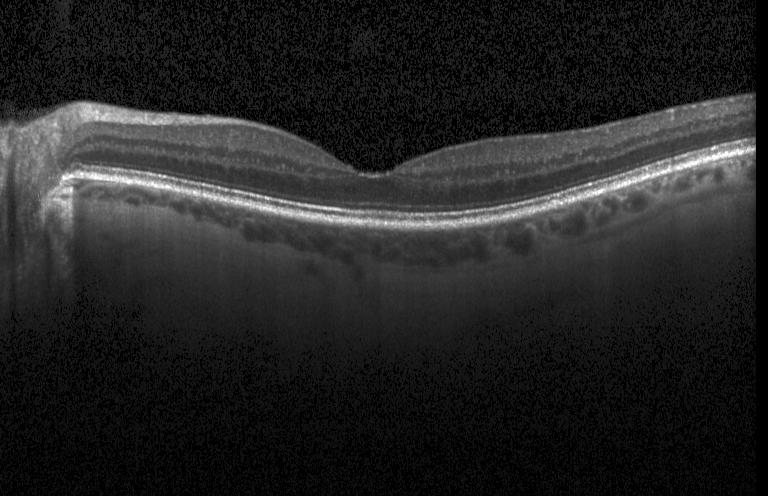
Dx: neither choroidal neovascularization, diabetic macular edema, nor drusen.